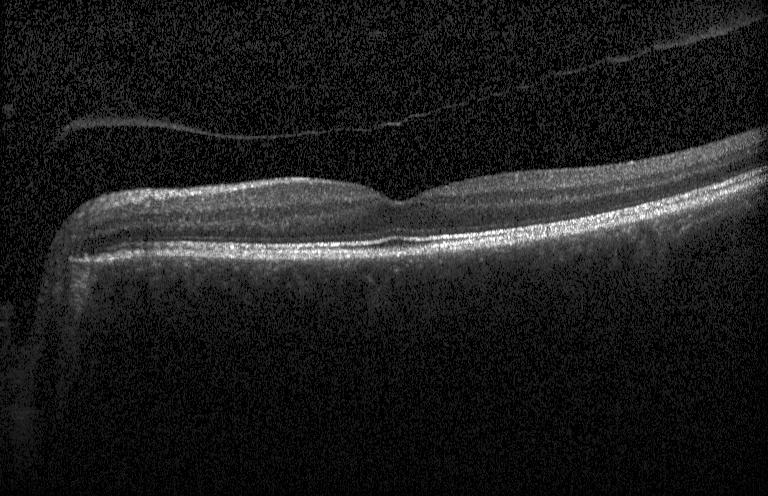

Heidelberg Spectralis. Retinal OCT B-scan. SD-OCT. Fovea-centered — Finding: no choroidal neovascularization, diabetic macular edema, or drusen.